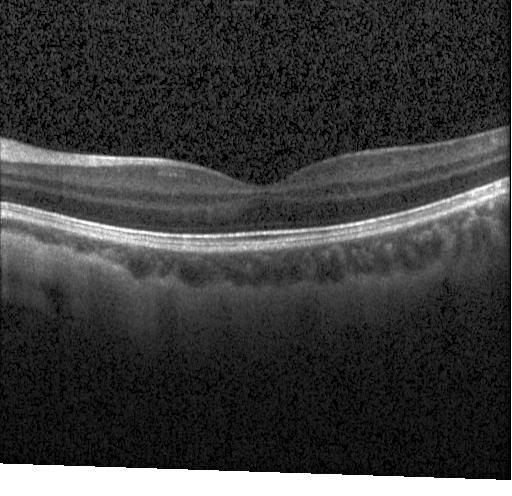

Heidelberg Spectralis · optical coherence tomography scan.
Impression: no choroidal neovascularization, no diabetic macular edema, and no drusen.